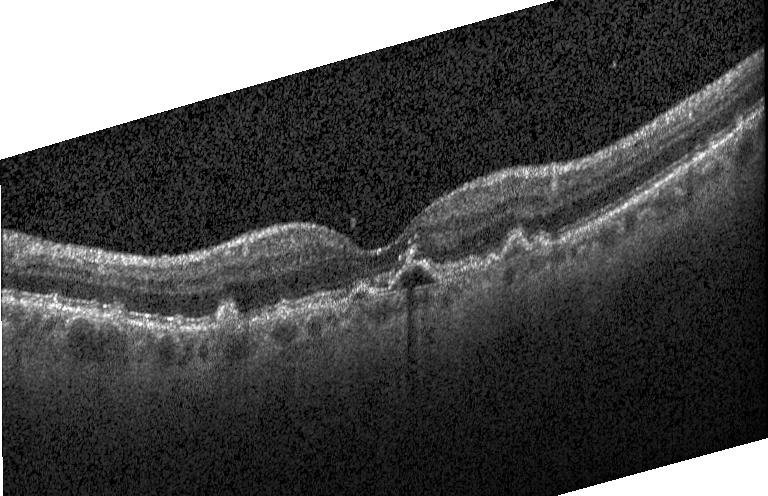

Finding: CNV.